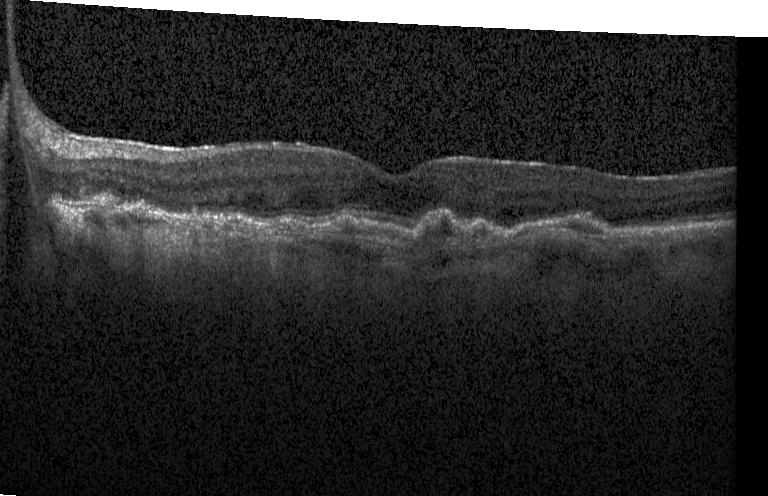
Retinal OCT B-scan — Macular OCT: a choroidal neovascular membrane.